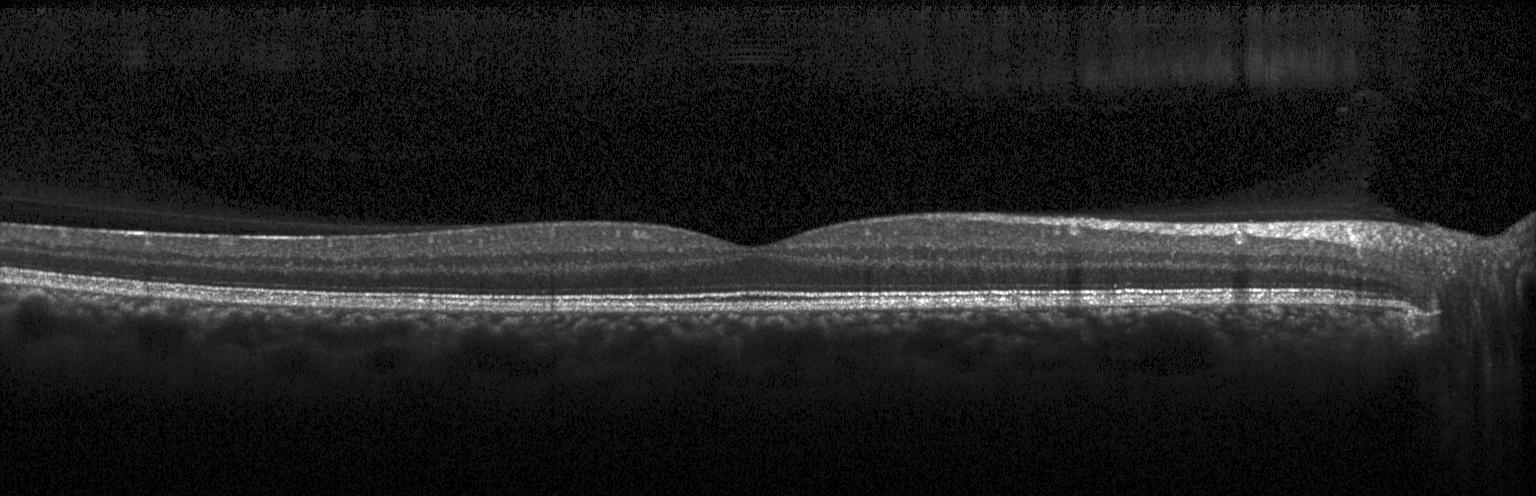 Finding: no CNV, no DME, and no drusen.